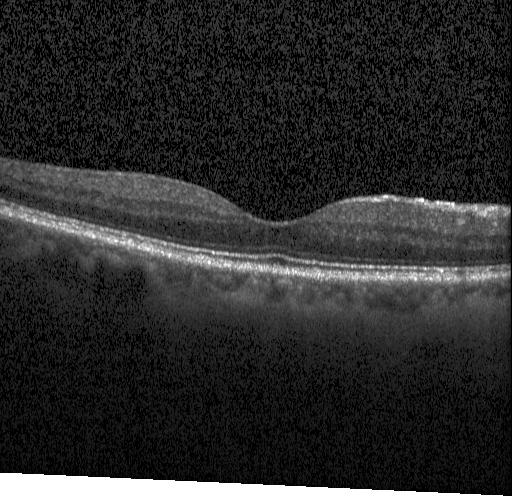
Optical coherence tomography scan, SD-OCT
Assessment: no evidence of choroidal neovascularization, diabetic macular edema, or drusen.